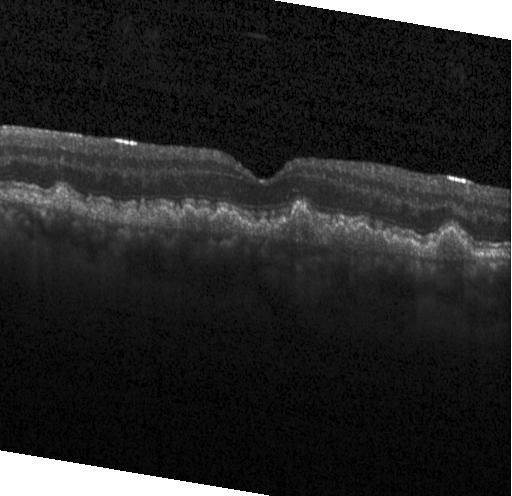 Spectral-domain optical coherence tomography; retinal OCT cross-section — OCT finding: a choroidal neovascular membrane.